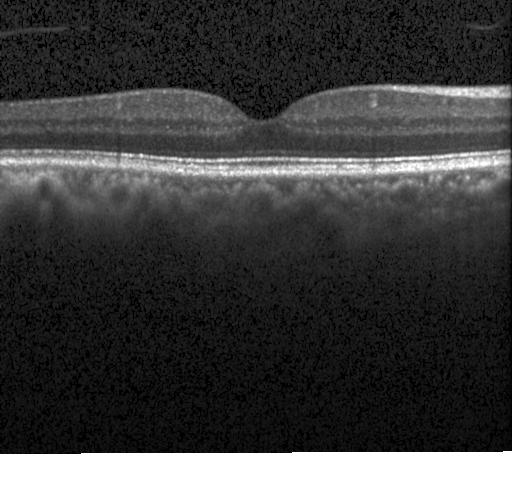 Retinal OCT cross-section — No CNV, no DME, and no drusen.